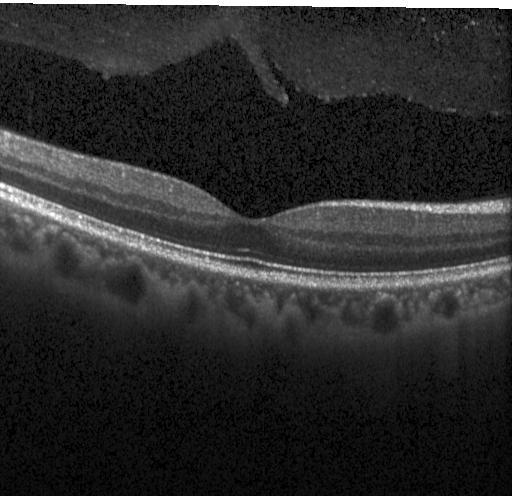 Centered on the fovea; optical coherence tomography scan — Diagnosis: no CNV, DME, or drusen.